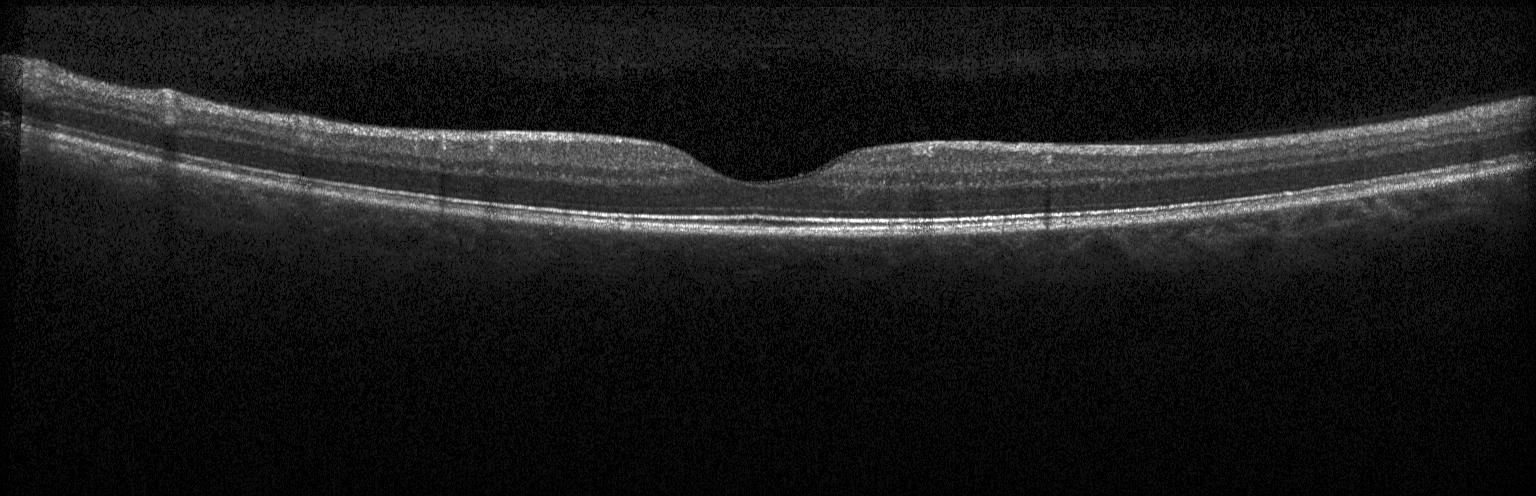

OCT B-scan — This B-scan demonstrates no choroidal neovascularization, diabetic macular edema, or drusen.